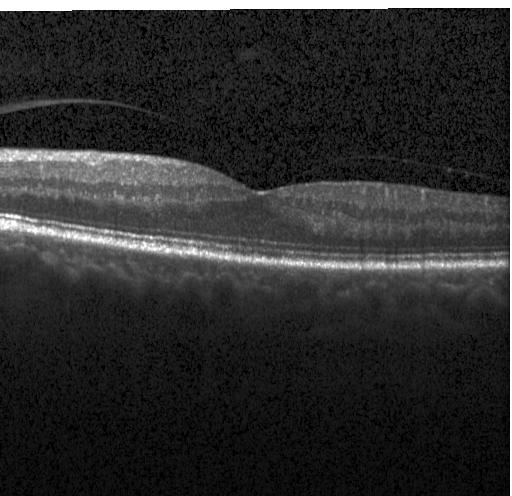

OCT B-scan; Heidelberg Spectralis; SD-OCT
Assessment: no evidence of choroidal neovascularization, diabetic macular edema, or drusen.